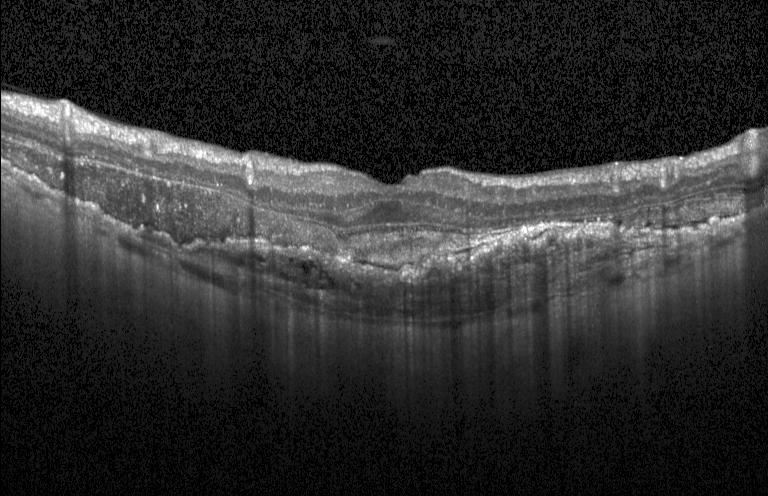
Dx: CNV.